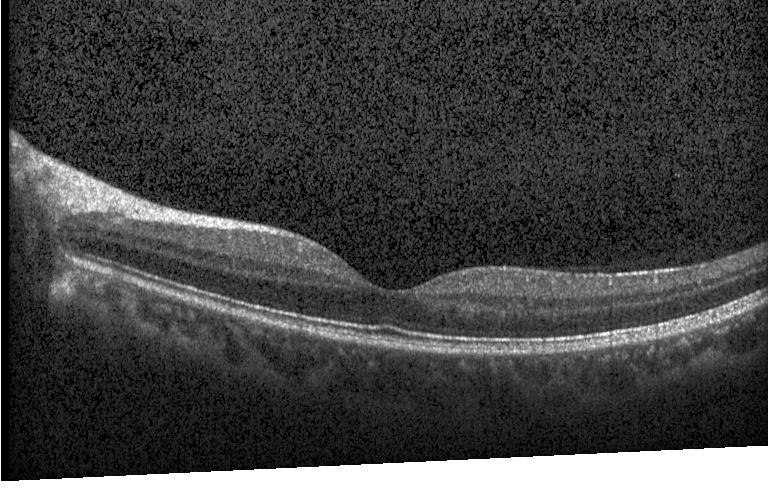 Retinal OCT B-scan. Finding: no choroidal neovascularization, no diabetic macular edema, and no drusen.